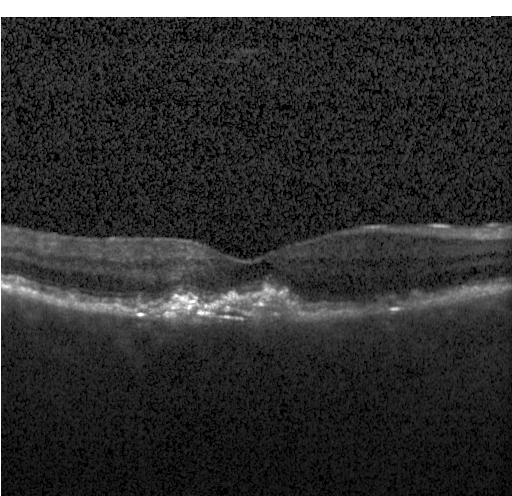 OCT line scan
Impression: CNV.